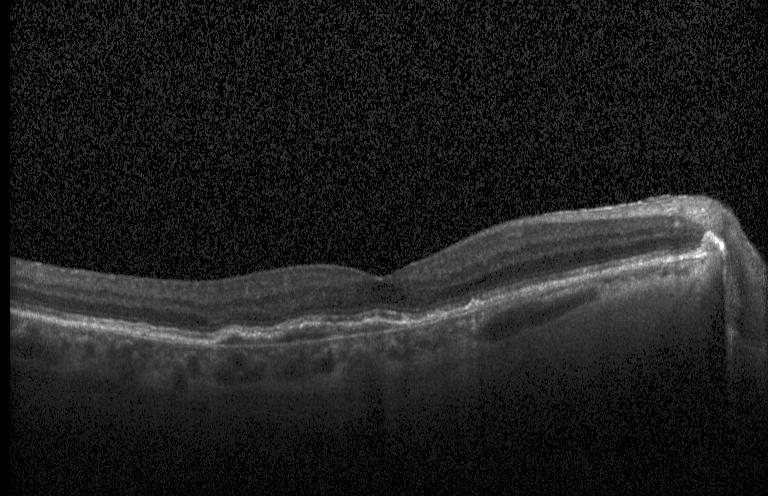
Macular OCT demonstrating choroidal neovascularization (CNV).